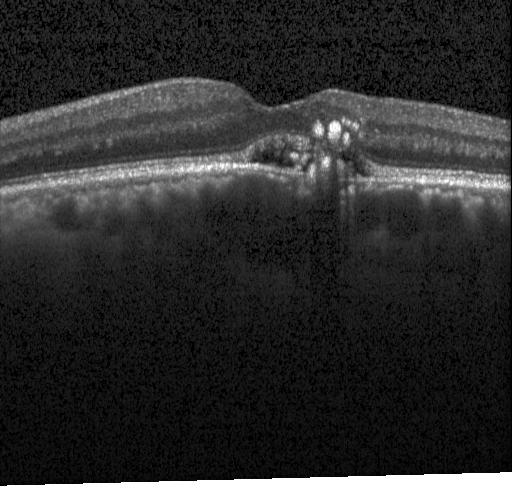 Macular scan. Spectral-domain OCT. Retinal OCT cross-section. Instrument: Heidelberg Spectralis — Macular OCT: choroidal neovascularization.